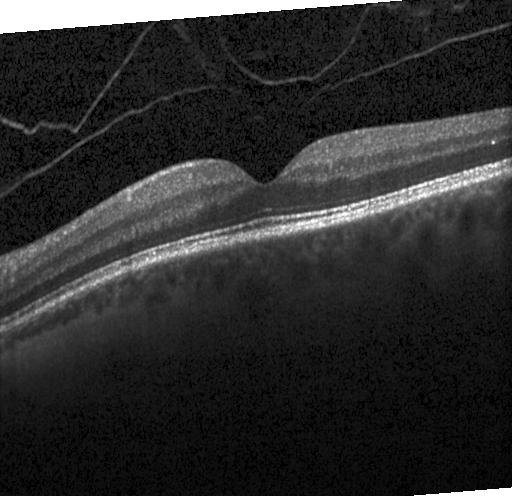

Centered on the fovea, instrument: Heidelberg Spectralis, OCT B-scan, spectral-domain optical coherence tomography — Finding: no CNV, DME, or drusen.